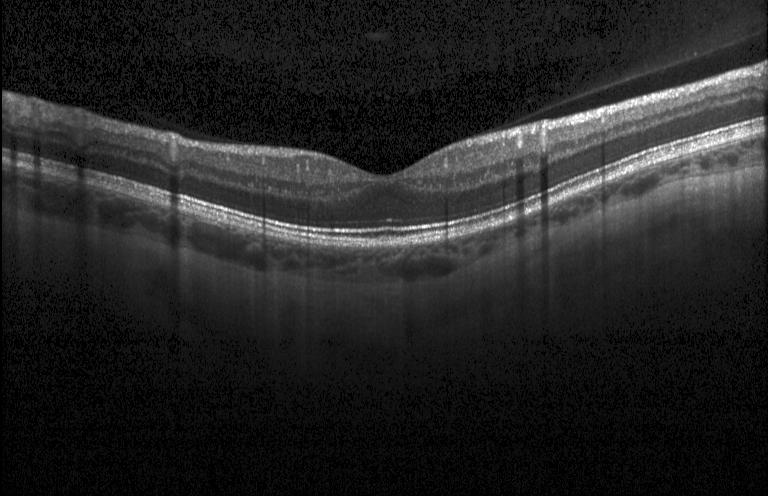 Spectral-domain optical coherence tomography, optical coherence tomography B-scan, instrument: Heidelberg Spectralis — Macular OCT: no choroidal neovascularization, diabetic macular edema, or drusen.